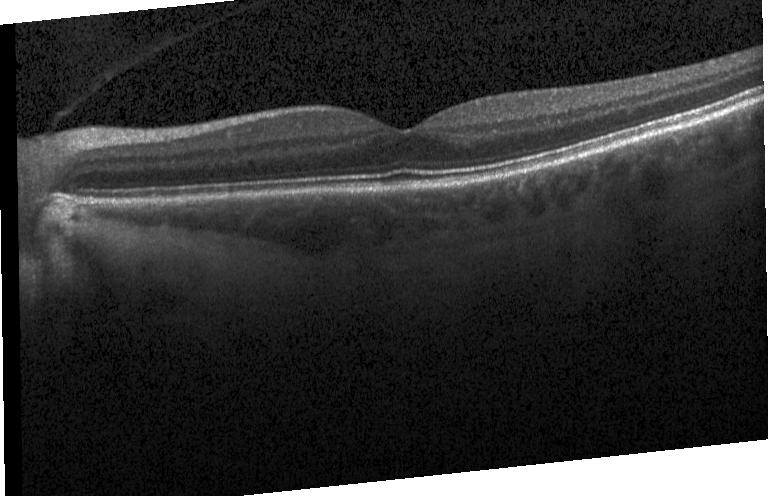 OCT B-scan showing no CNV, no DME, and no drusen.